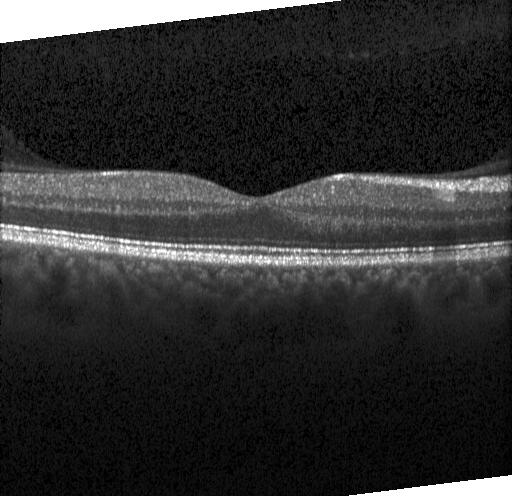
Centered on the fovea. Retinal OCT cross-section. Spectral-domain optical coherence tomography — No CNV, DME, or drusen.